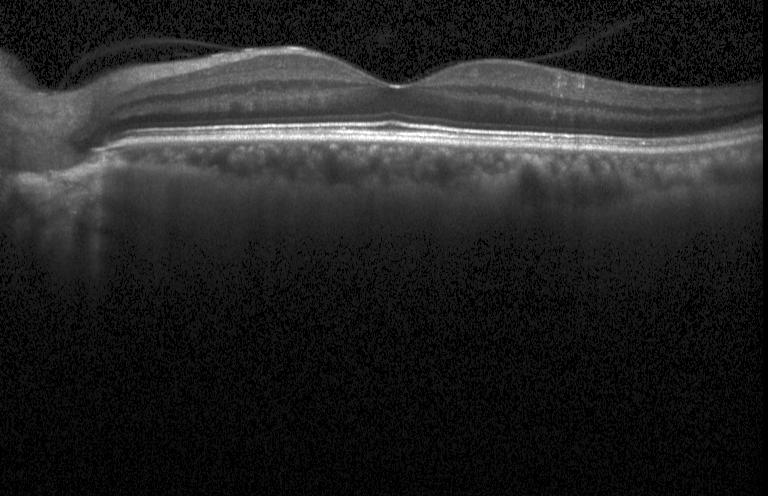 Fovea-centered; spectral-domain OCT; optical coherence tomography scan; Heidelberg Spectralis
Finding: no evidence of choroidal neovascularization, diabetic macular edema, or drusen.